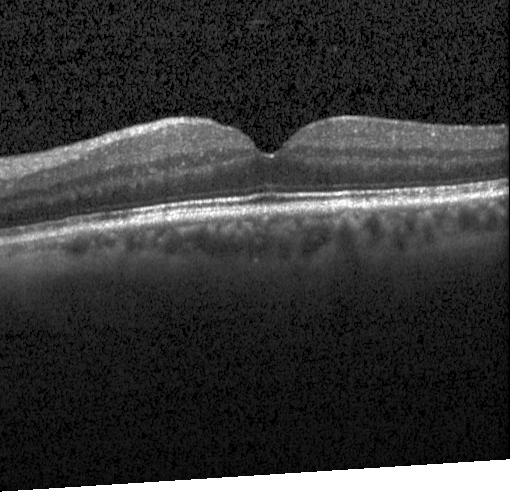

Retinal OCT B-scan; spectral-domain OCT; macular scan; Heidelberg Spectralis OCT system. OCT finding: neither choroidal neovascularization, diabetic macular edema, nor drusen.